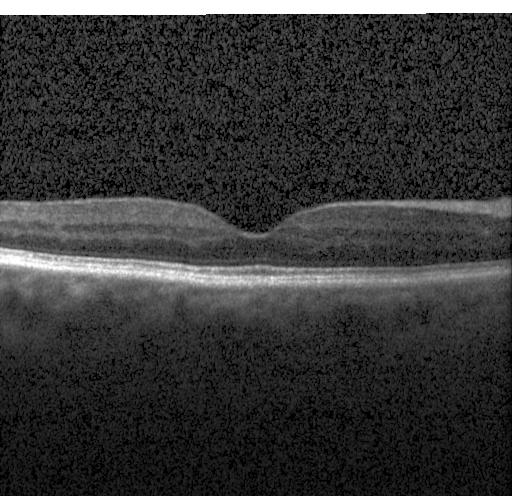

Finding: no choroidal neovascularization, diabetic macular edema, or drusen.